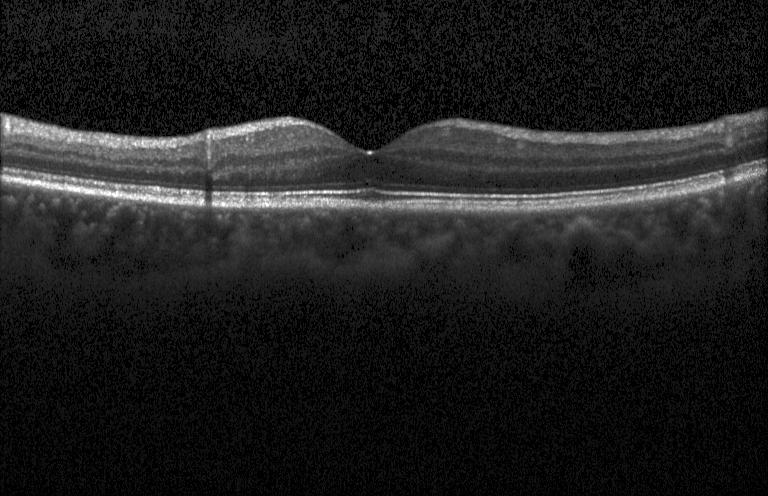
OCT B-scan; macular scan. Diagnosis: neither CNV, DME, nor drusen.